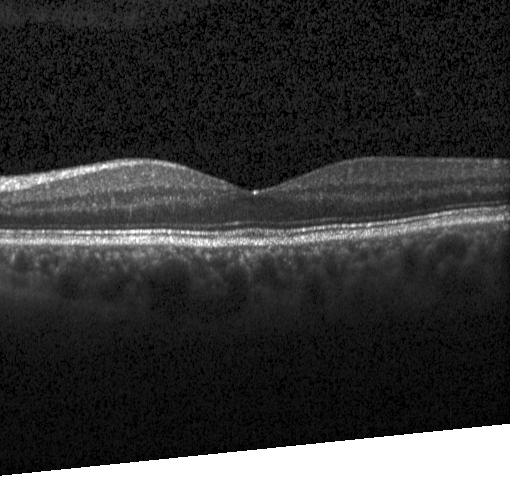 Retinal OCT cross-section.
OCT finding: neither choroidal neovascularization, diabetic macular edema, nor drusen.